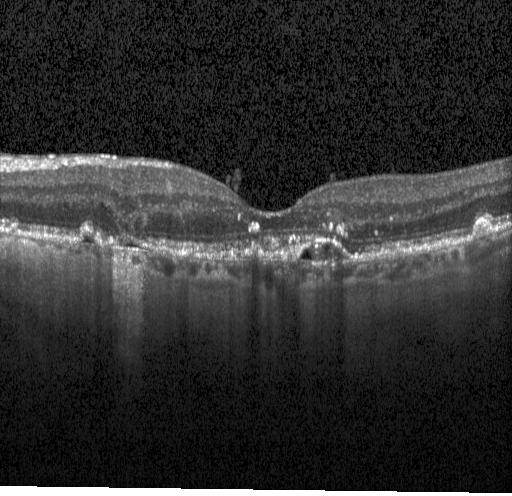 OCT line scan; Heidelberg Spectralis; horizontal scan through the fovea — Impression: CNV.